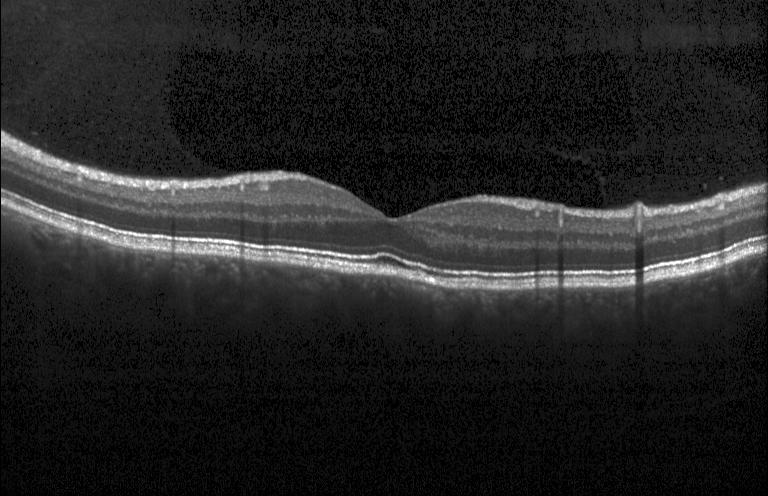
Neither choroidal neovascularization, diabetic macular edema, nor drusen.